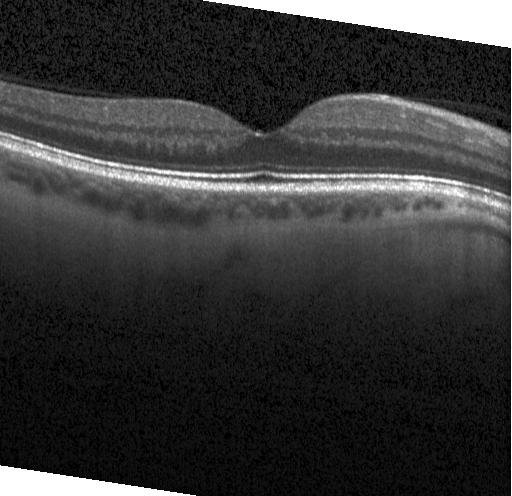
Retinal OCT B-scan — Assessment: no evidence of choroidal neovascularization, diabetic macular edema, or drusen.